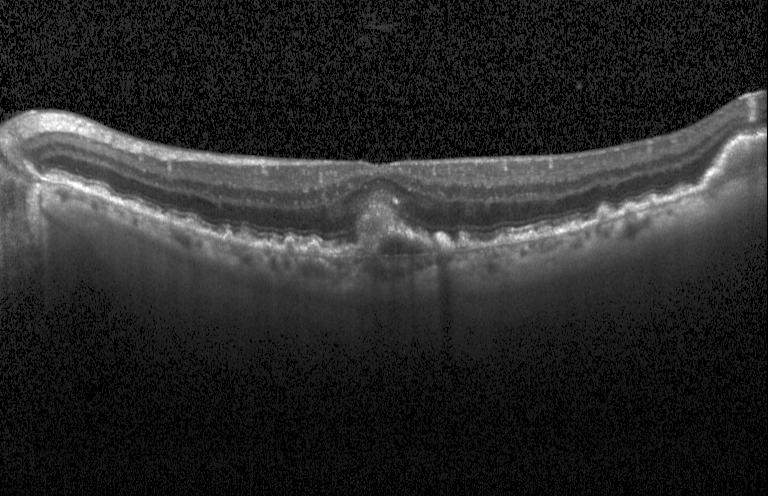 Optical coherence tomography scan · spectral-domain optical coherence tomography · Heidelberg Spectralis. Finding: CNV.